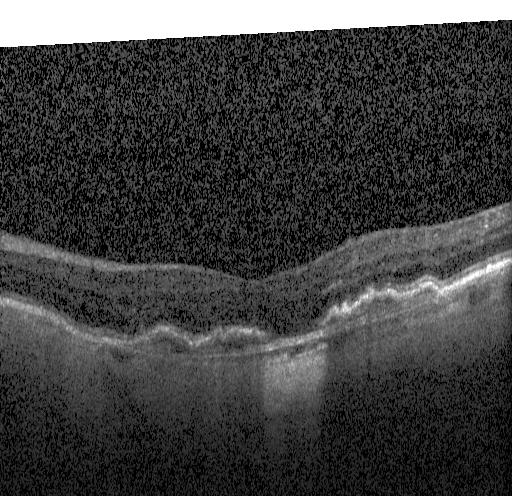 Acquired on a Heidelberg Spectralis, OCT B-scan, through the macula, spectral-domain OCT. The scan shows a choroidal neovascular membrane.